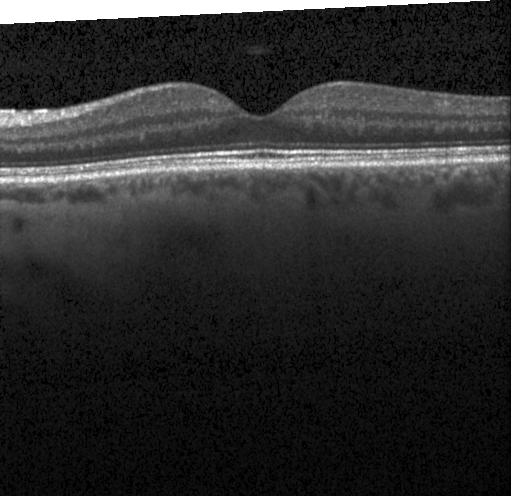 Fovea-centered; OCT line scan; Heidelberg Spectralis; spectral-domain optical coherence tomography.
OCT finding: no evidence of choroidal neovascularization, diabetic macular edema, or drusen.